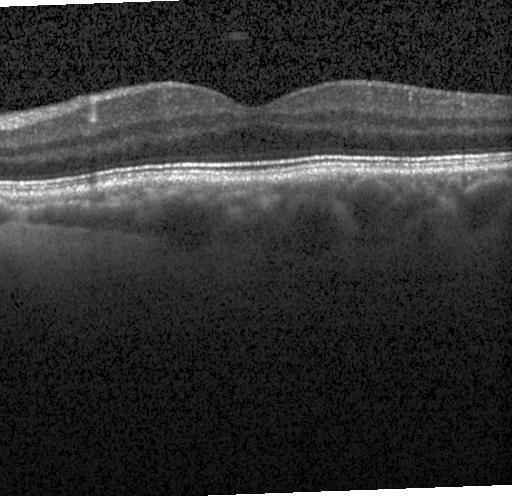

Instrument: Heidelberg Spectralis. Retinal OCT cross-section. SD-OCT — Assessment: neither choroidal neovascularization, diabetic macular edema, nor drusen.